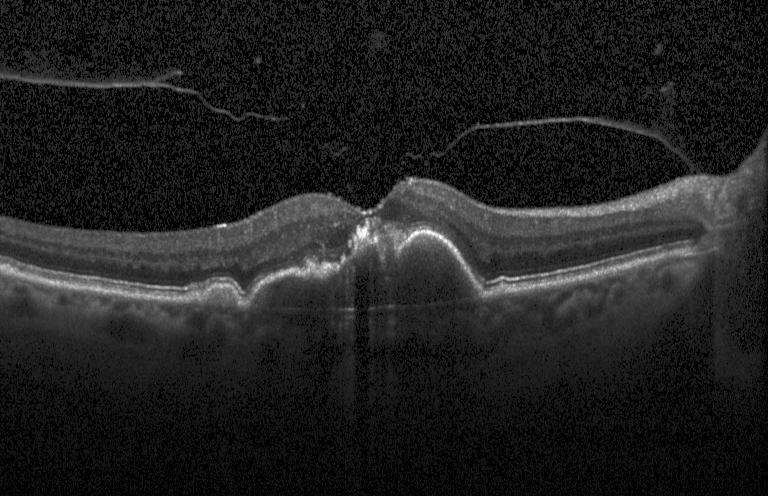

OCT line scan.
Diagnosis: choroidal neovascularization.